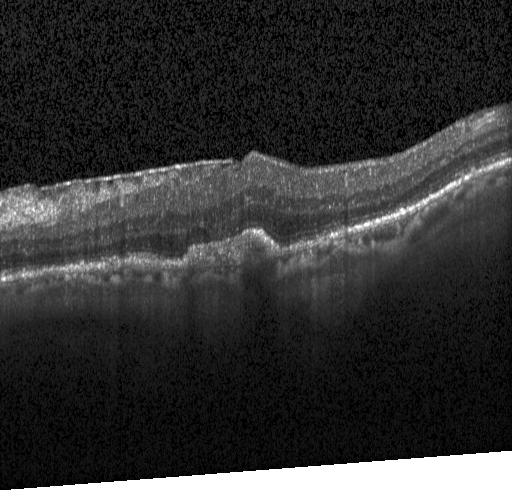
Macular scan, optical coherence tomography scan, Heidelberg Spectralis OCT system.
Diagnosis: choroidal neovascularization.